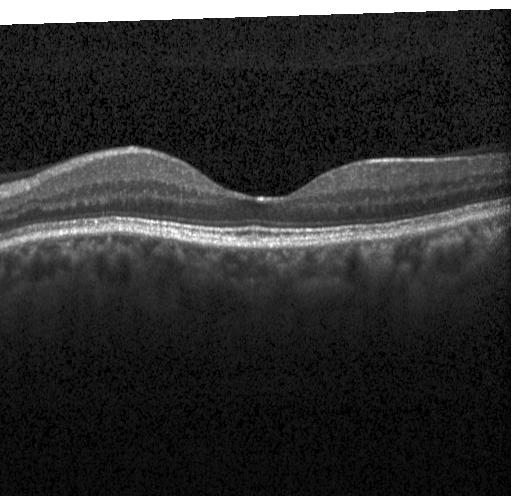
Optical coherence tomography scan
Diagnosis: no choroidal neovascularization, diabetic macular edema, or drusen.